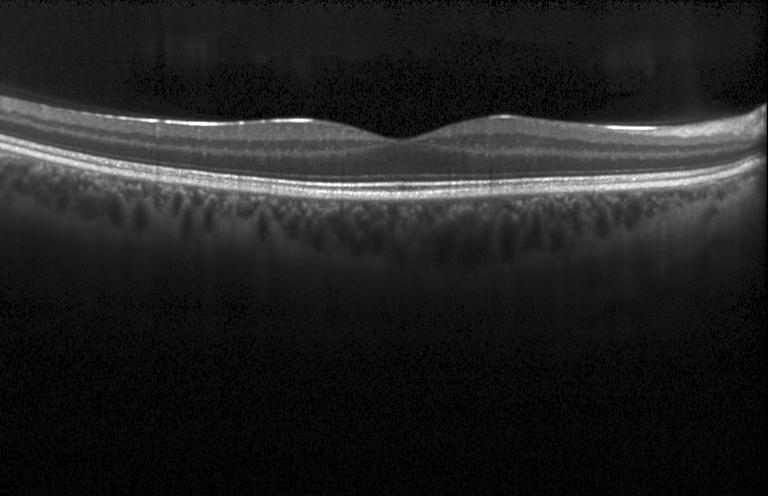
Dx: no evidence of choroidal neovascularization, diabetic macular edema, or drusen.